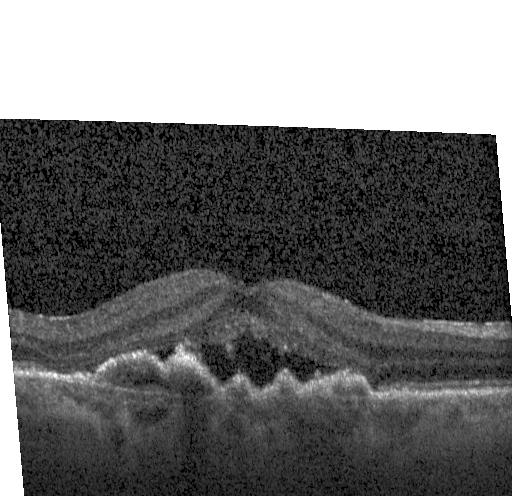 Instrument: Heidelberg Spectralis; centered on the fovea; OCT line scan — Impression: a choroidal neovascular membrane.